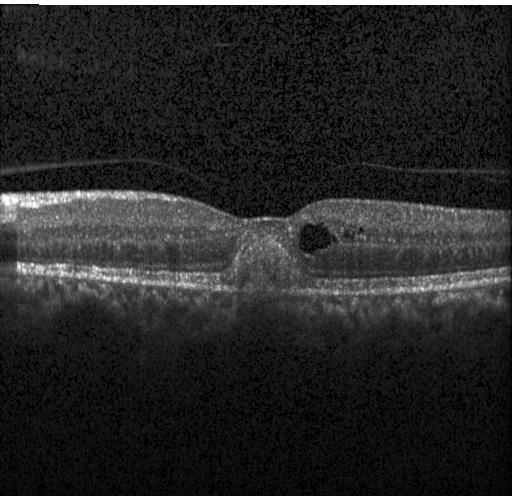 Optical coherence tomography scan, Heidelberg Spectralis OCT system — Impression: choroidal neovascularization.